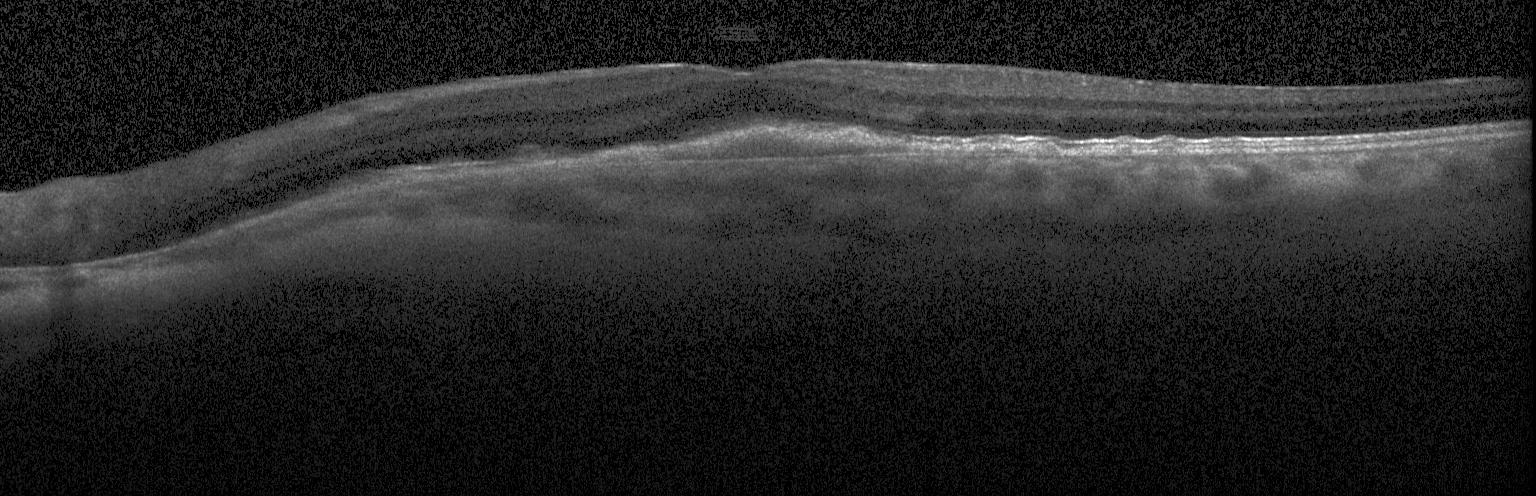

Instrument: Heidelberg Spectralis; centered on the fovea; spectral-domain optical coherence tomography; optical coherence tomography scan — Diagnosis: a choroidal neovascular membrane.